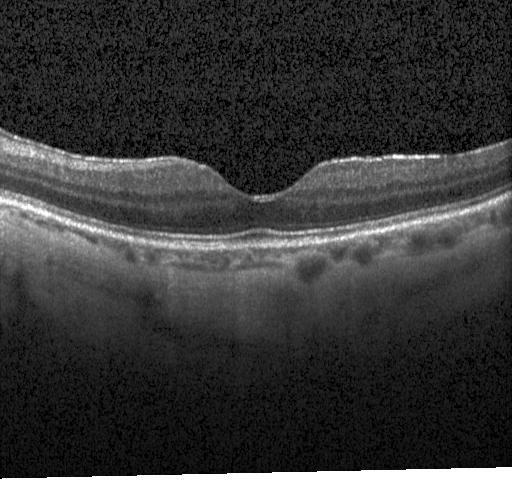

Optical coherence tomography scan, horizontal scan through the fovea. No choroidal neovascularization, diabetic macular edema, or drusen.